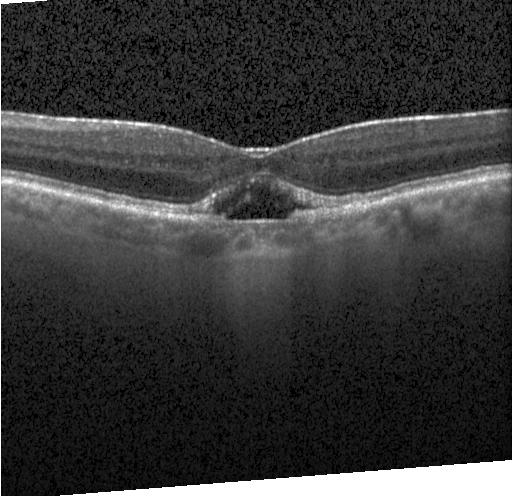

A choroidal neovascular membrane.